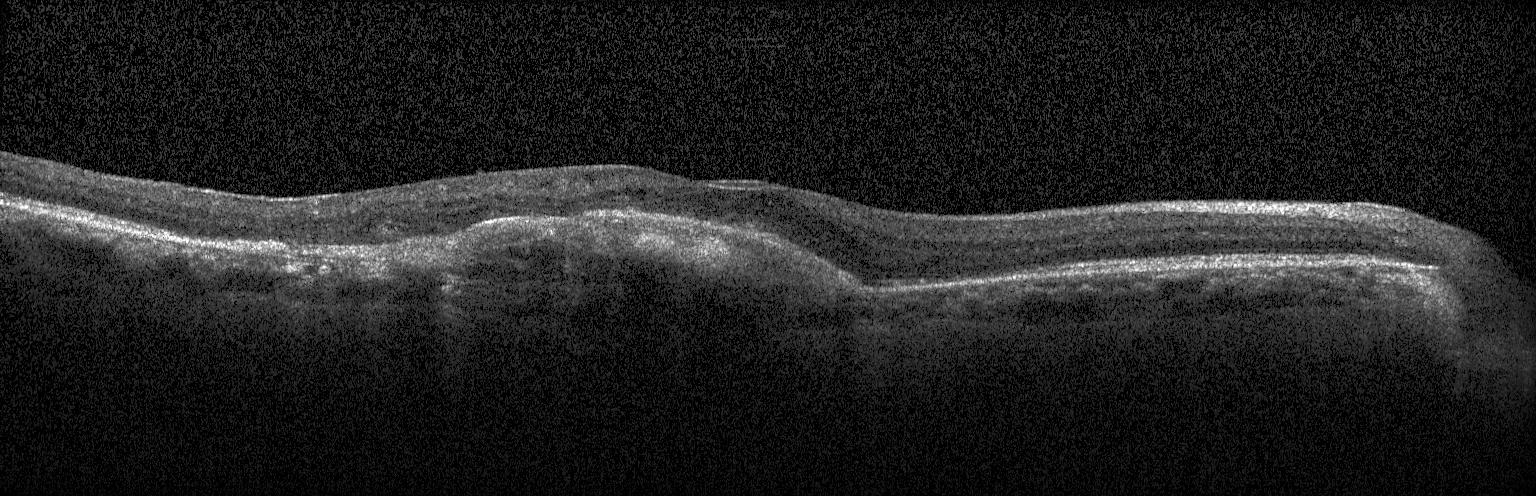

Fovea-centered, Heidelberg Spectralis, OCT line scan, spectral-domain optical coherence tomography
Dx: CNV.